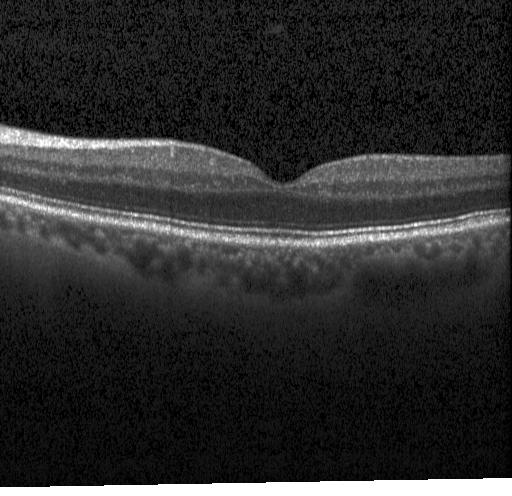 Spectral-domain OCT · centered on the fovea · retinal OCT B-scan
Diagnosis: no CNV, DME, or drusen.